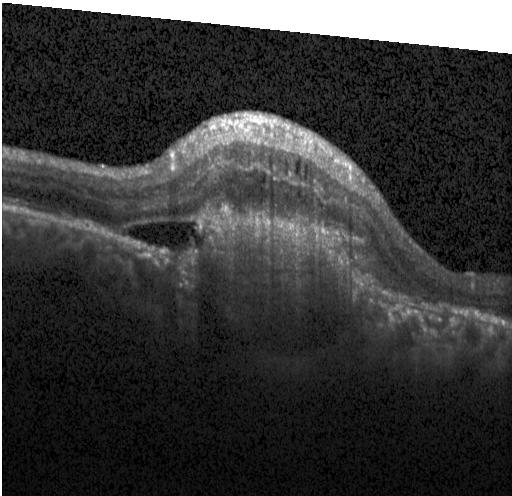
OCT line scan.
Diagnosis: choroidal neovascularization (CNV).